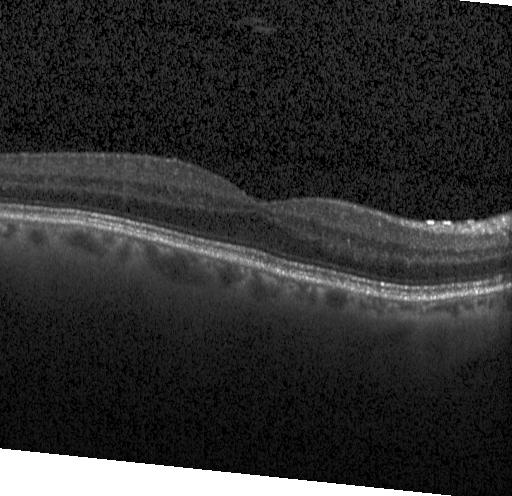 Through the macula, SD-OCT, retinal OCT B-scan.
Neither choroidal neovascularization, diabetic macular edema, nor drusen.